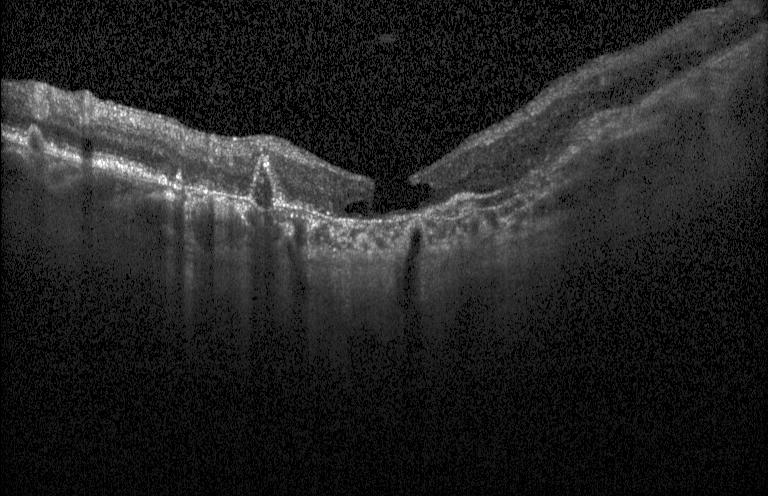
Retinal OCT B-scan. Heidelberg Spectralis. Spectral-domain OCT
Assessment: a choroidal neovascular membrane.